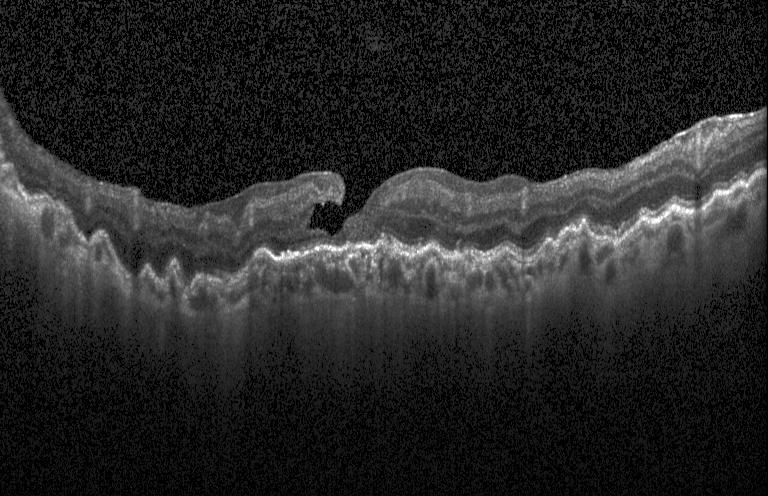

OCT B-scan showing a choroidal neovascular membrane.